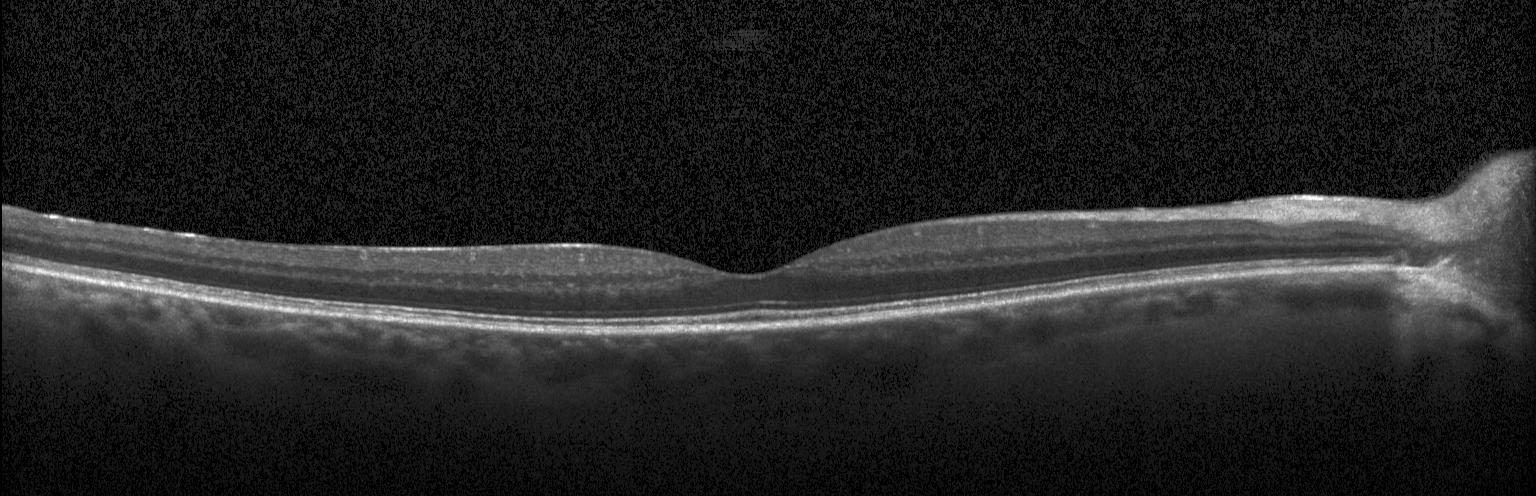

Horizontal scan through the fovea; Heidelberg Spectralis; optical coherence tomography scan; spectral-domain OCT
Assessment: neither choroidal neovascularization, diabetic macular edema, nor drusen.